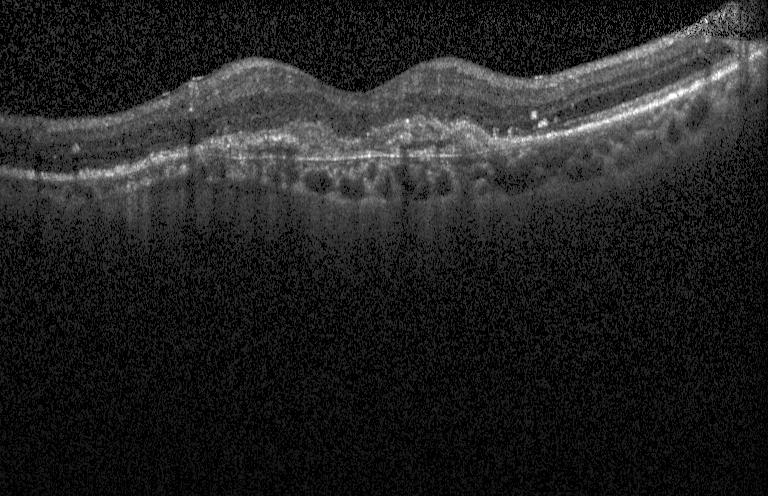 OCT B-scan showing a choroidal neovascular membrane.